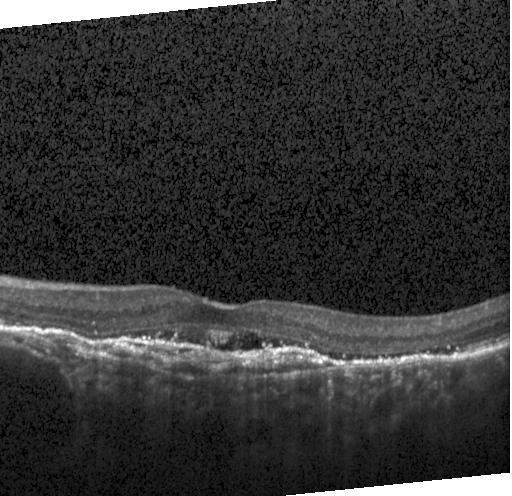 Retinal OCT cross-section · SD-OCT.
The scan shows choroidal neovascularization.